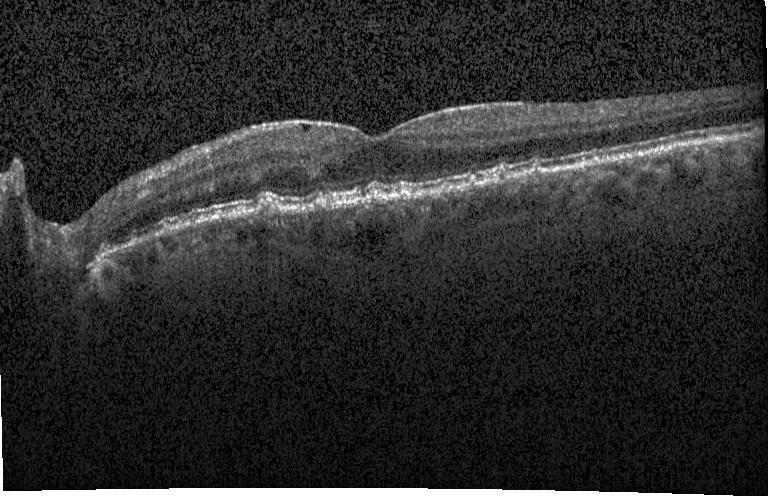

SD-OCT. Fovea-centered. OCT B-scan — OCT finding: multiple drusen.